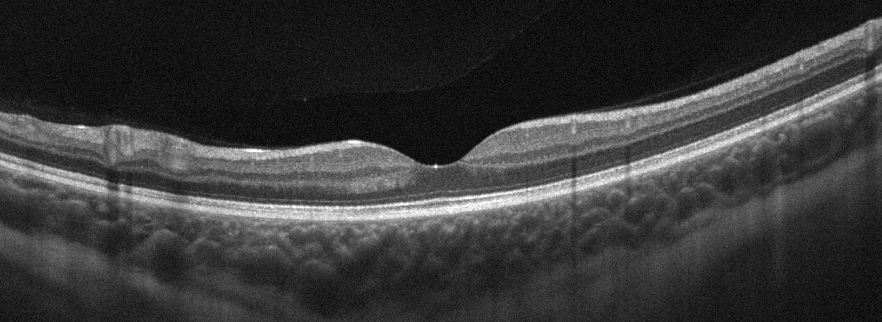 Through the macula, retinal OCT cross-section, instrument: Optovue Avanti RTVue XR — Assessment: absence of AMD, DME, ERM, RAO, RVO, and vitreomacular interface disease.